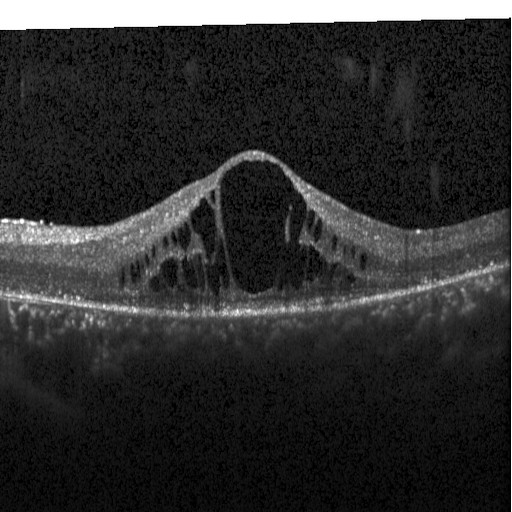

Optical coherence tomography scan.
The scan shows DME.